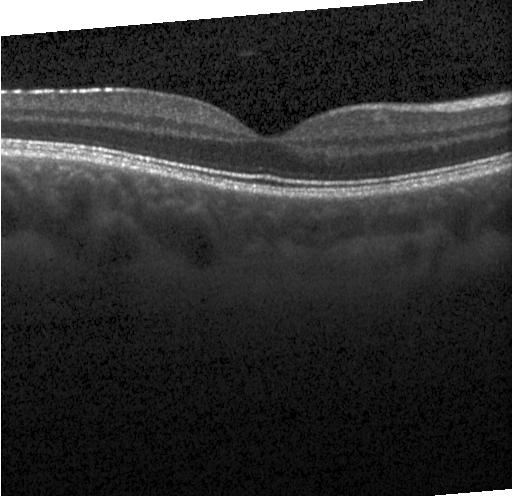

Optical coherence tomography B-scan; instrument: Heidelberg Spectralis; horizontal scan through the fovea. Macular OCT: no evidence of choroidal neovascularization, diabetic macular edema, or drusen.